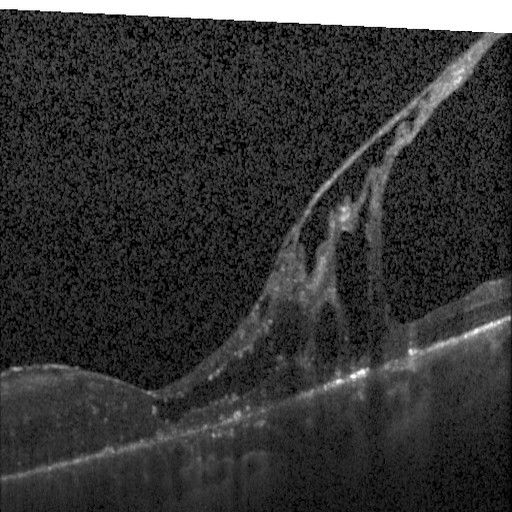 OCT B-scan showing diabetic macular edema.